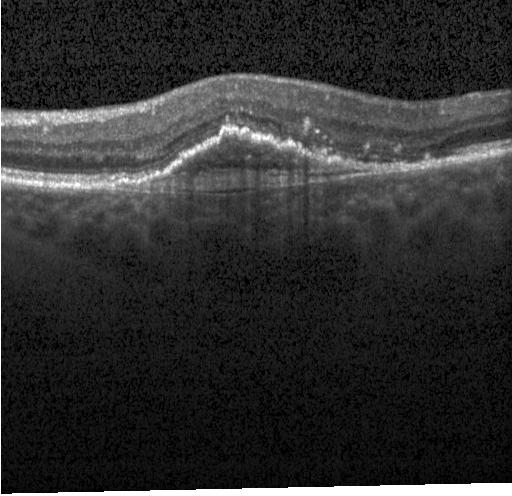 Optical coherence tomography scan · Heidelberg Spectralis.
Impression: a choroidal neovascular membrane.